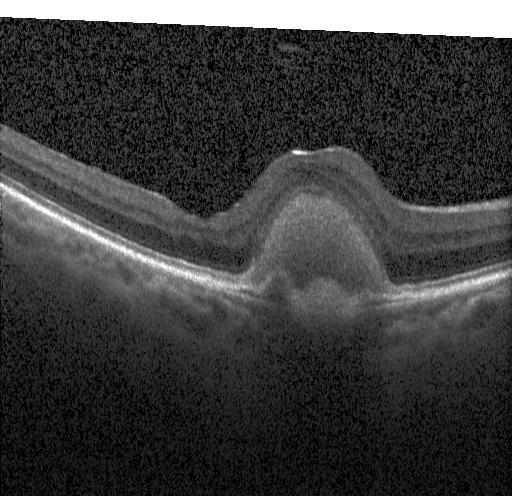
Centered on the fovea; SD-OCT; instrument: Heidelberg Spectralis; optical coherence tomography B-scan — OCT finding: a choroidal neovascular membrane.